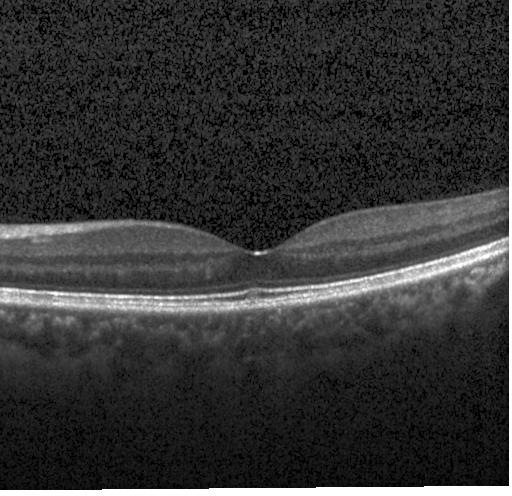 This B-scan demonstrates no evidence of choroidal neovascularization, diabetic macular edema, or drusen.